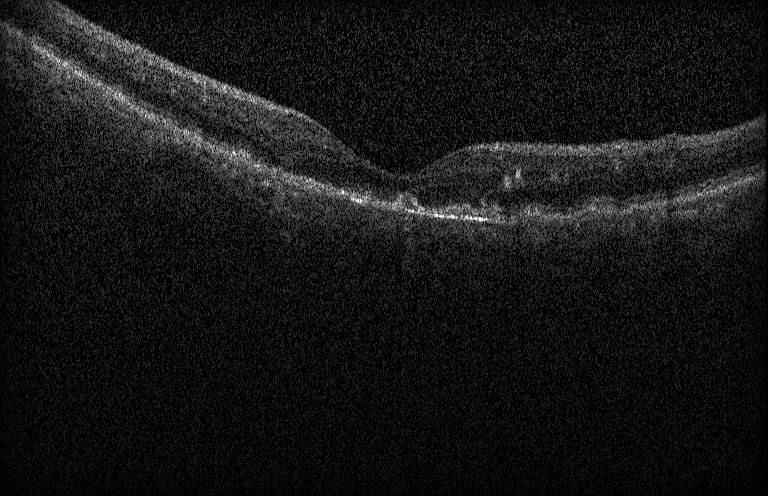

Optical coherence tomography B-scan. Spectral-domain OCT. Instrument: Heidelberg Spectralis. Choroidal neovascularization.